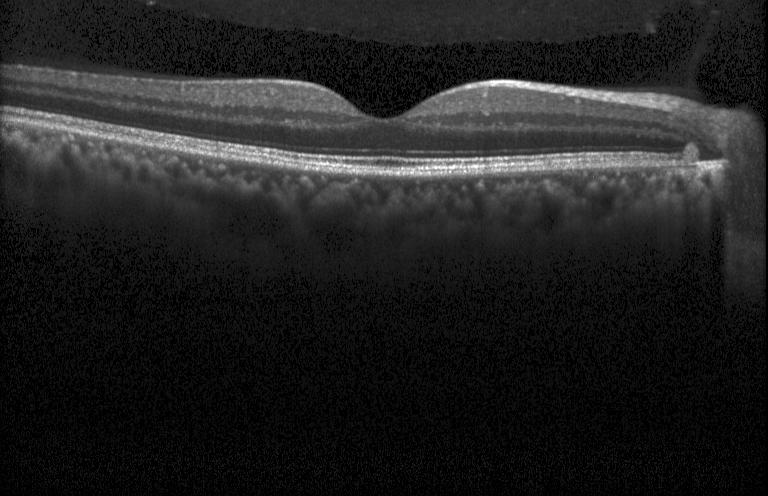
Retinal OCT B-scan — Finding: no choroidal neovascularization, no diabetic macular edema, and no drusen.